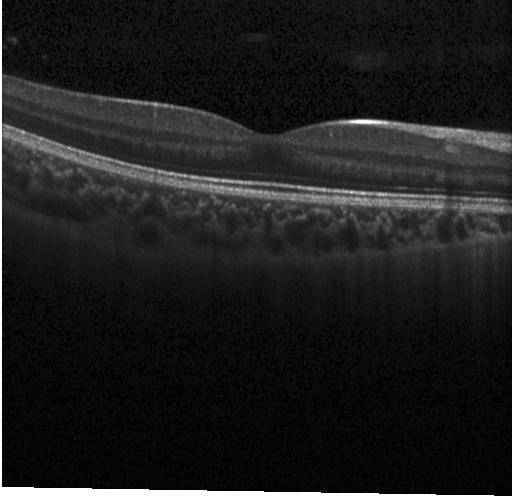

Diagnosis: no CNV, no DME, and no drusen.